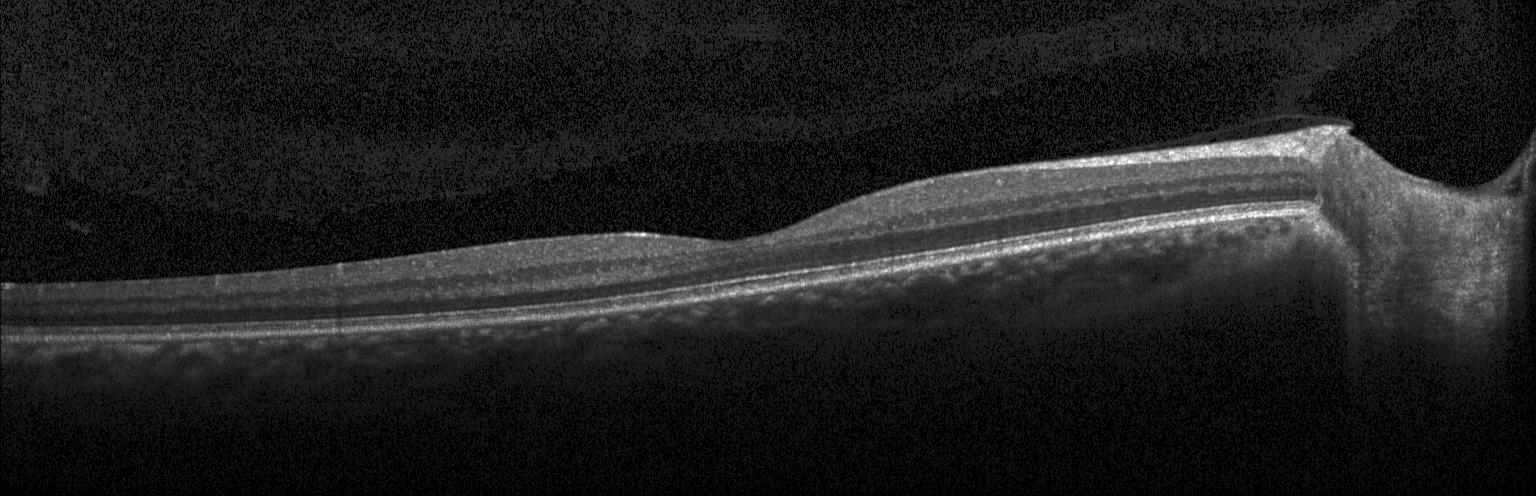 Optical coherence tomography scan. Spectral-domain OCT. Macular scan
The scan shows no evidence of choroidal neovascularization, diabetic macular edema, or drusen.